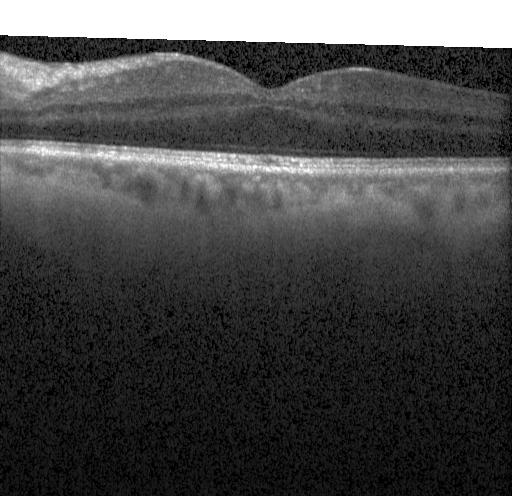 Assessment: no evidence of CNV, DME, or drusen.